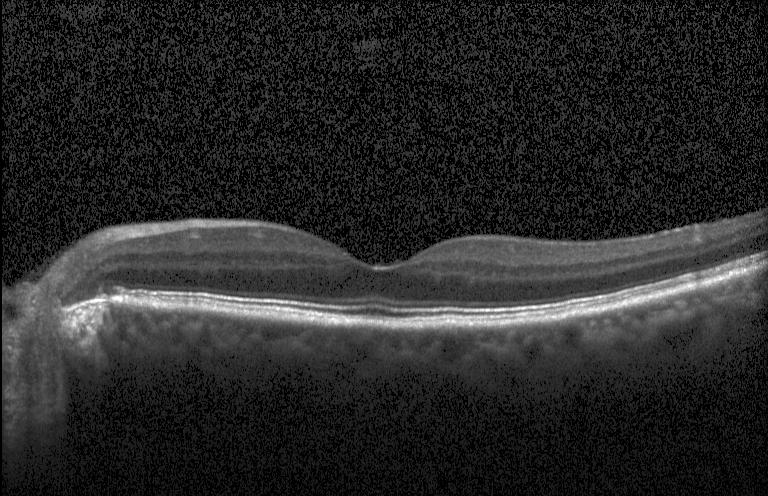 OCT line scan. Through the macula.
Diagnosis: neither CNV, DME, nor drusen.